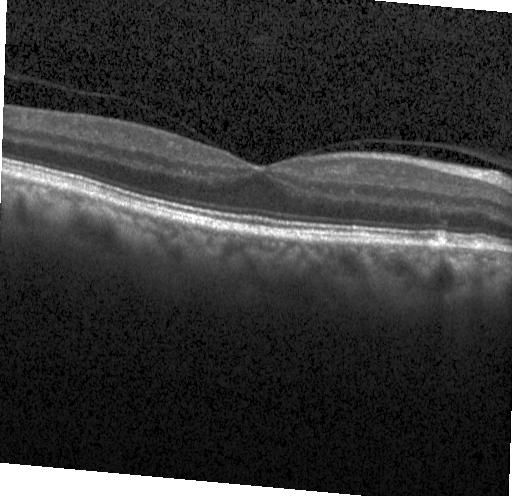 Macular scan, optical coherence tomography B-scan, spectral-domain OCT.
Impression: multiple drusen.